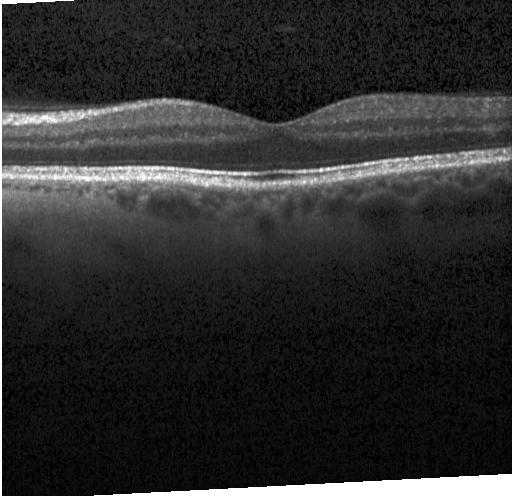
Optical coherence tomography scan; Heidelberg Spectralis OCT system; through the macula; spectral-domain OCT. The scan shows no choroidal neovascularization, no diabetic macular edema, and no drusen.